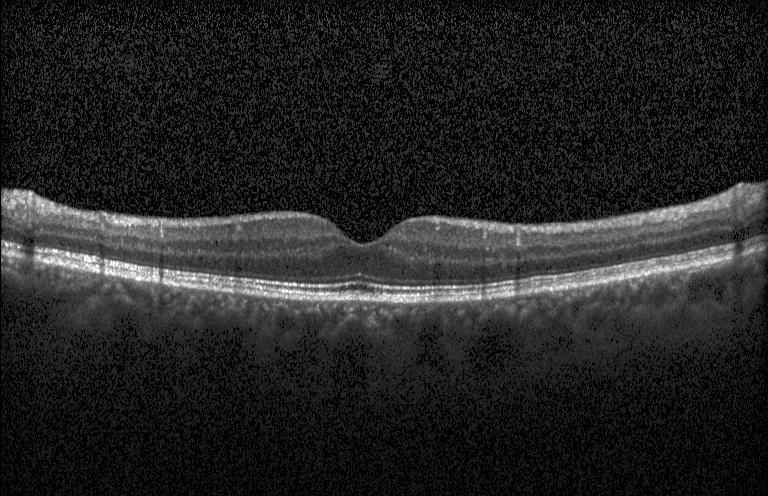
Impression: neither choroidal neovascularization, diabetic macular edema, nor drusen.